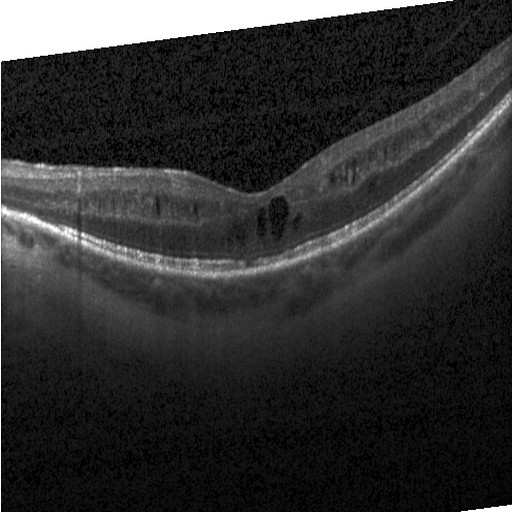
OCT B-scan. Spectral-domain OCT. Heidelberg Spectralis OCT system. Diabetic macular edema (DME).